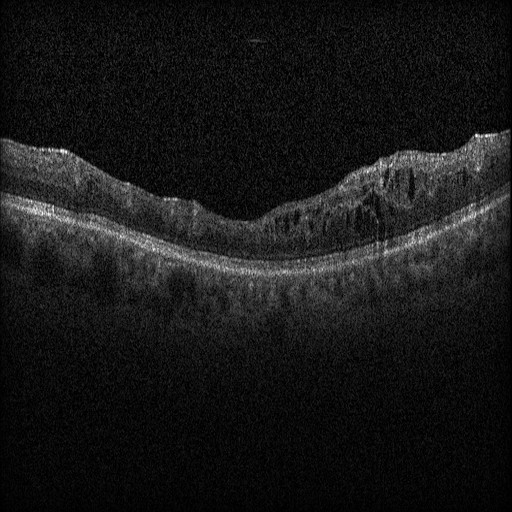

OCT B-scan showing DME.